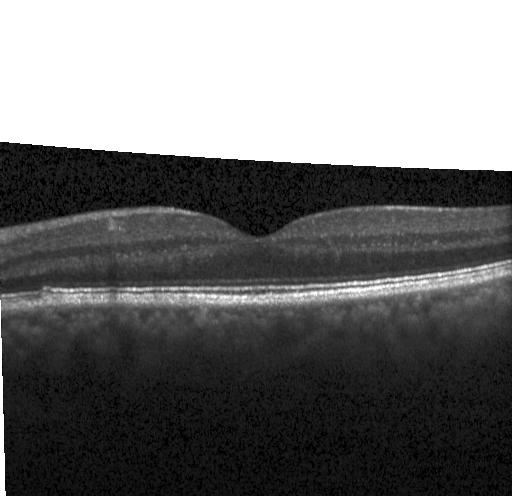
Retinal OCT cross-section showing no choroidal neovascularization, no diabetic macular edema, and no drusen.